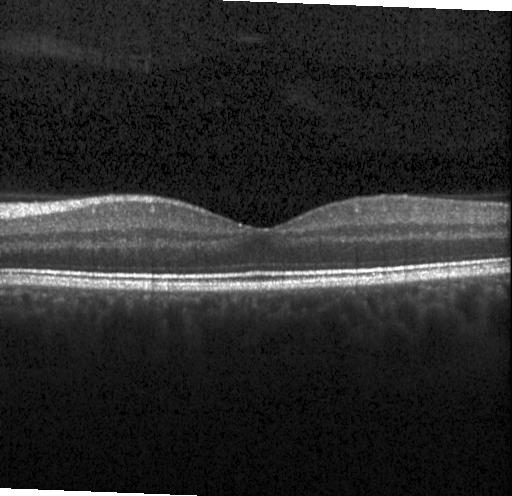 OCT line scan
Dx: no evidence of CNV, DME, or drusen.